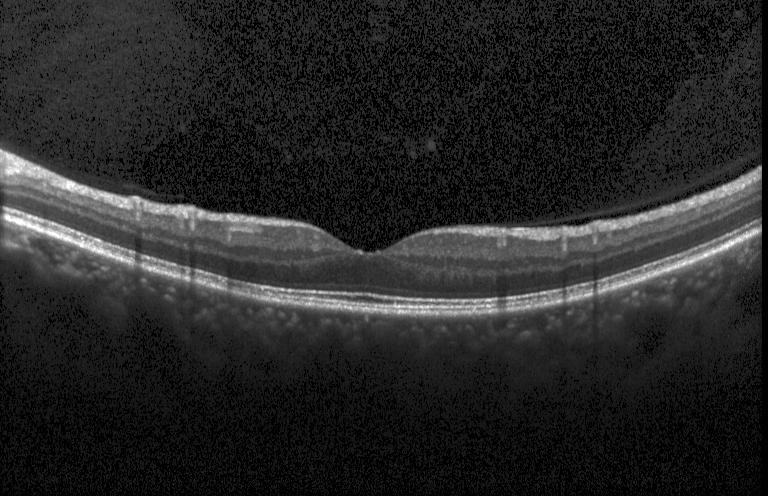
Spectral-domain OCT B-scan: no evidence of choroidal neovascularization, diabetic macular edema, or drusen.